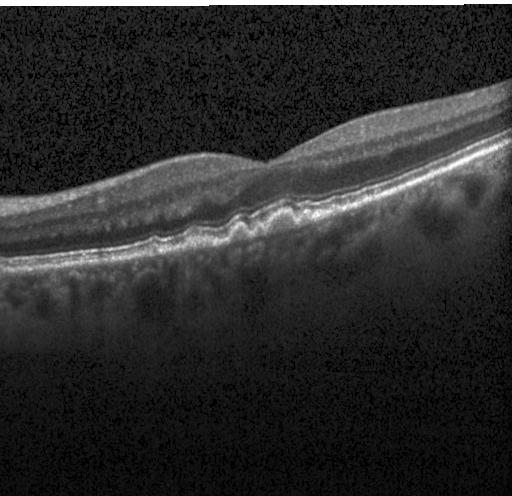

Heidelberg Spectralis OCT system. Centered on the fovea. Retinal OCT cross-section. Assessment: drusen.